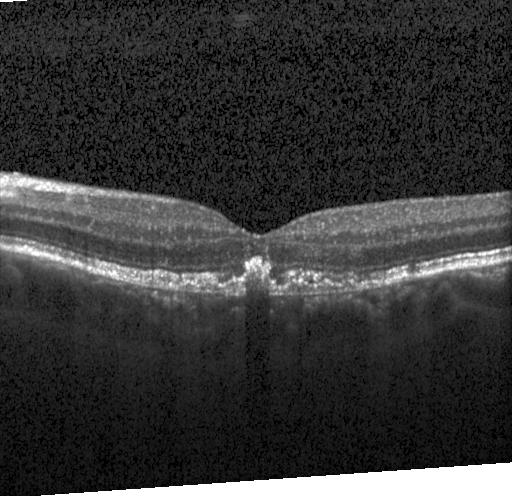

Heidelberg Spectralis. OCT B-scan. Through the macula. SD-OCT — Assessment: choroidal neovascularization (CNV).